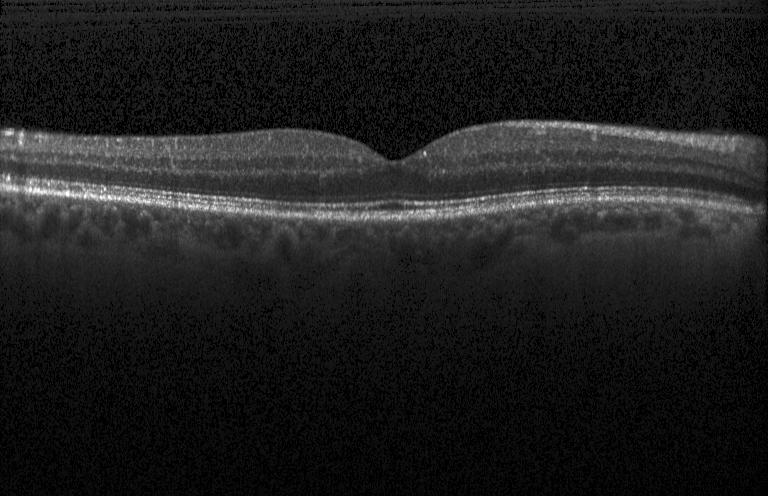
Fovea-centered. Spectral-domain OCT. Retinal OCT cross-section — OCT finding: no choroidal neovascularization, no diabetic macular edema, and no drusen.